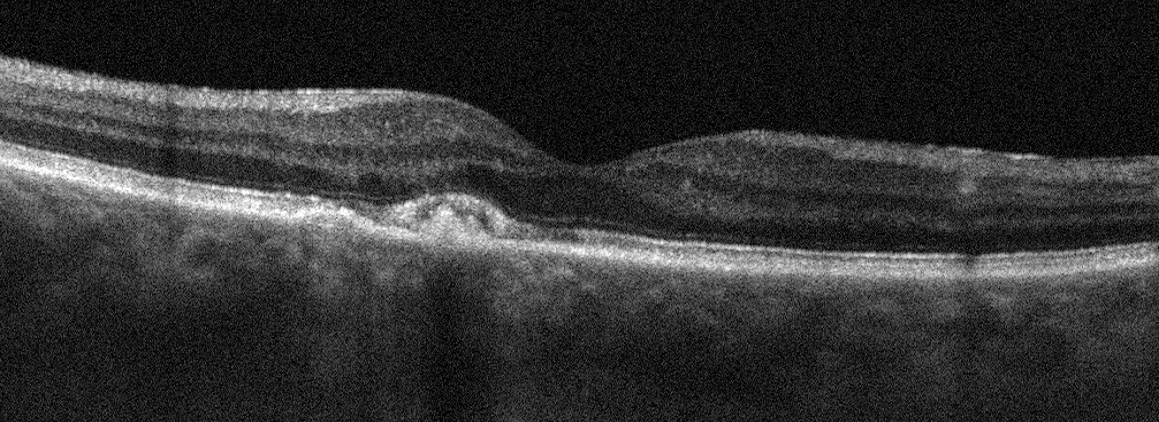
Oculus sinister. Retinal OCT B-scan
Assessment: AMD.